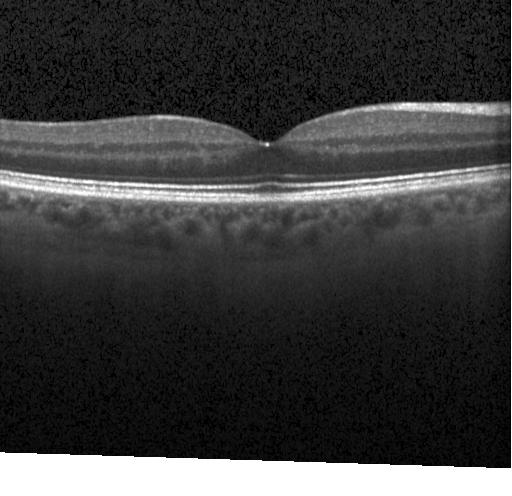 Finding: no evidence of choroidal neovascularization, diabetic macular edema, or drusen.